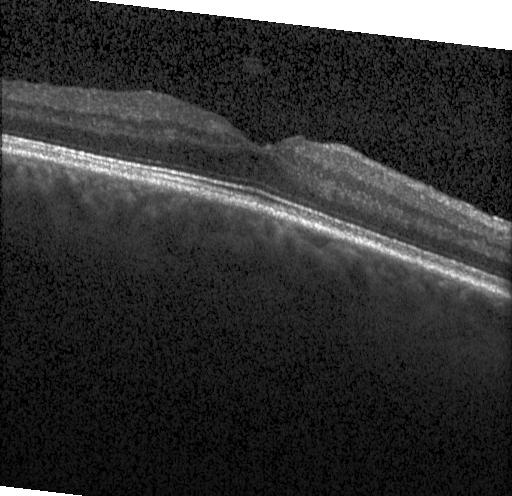 Spectral-domain OCT B-scan: no choroidal neovascularization, no diabetic macular edema, and no drusen.